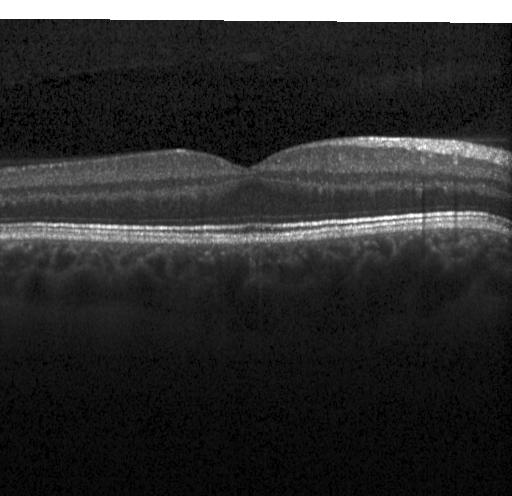
Spectral-domain OCT B-scan: no choroidal neovascularization, diabetic macular edema, or drusen.